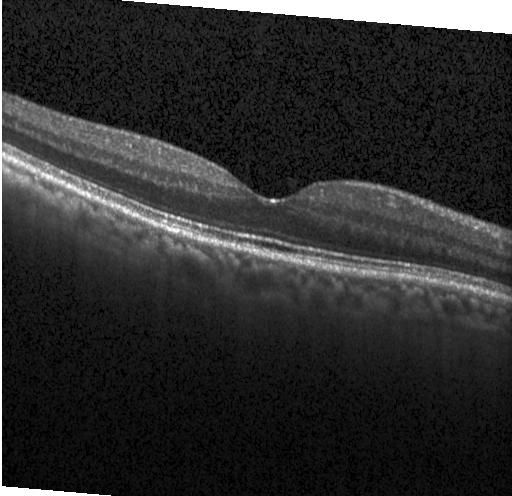

Optical coherence tomography scan. Diagnosis: no choroidal neovascularization, no diabetic macular edema, and no drusen.